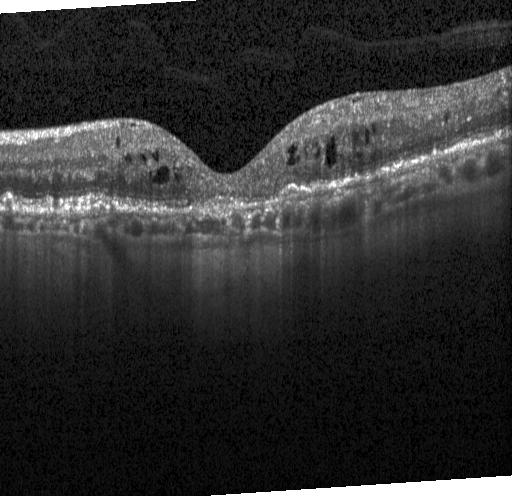
OCT B-scan — The scan shows a choroidal neovascular membrane.